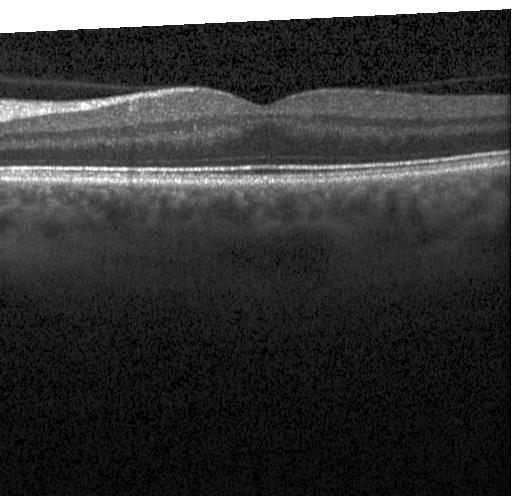 The scan shows no choroidal neovascularization, no diabetic macular edema, and no drusen.